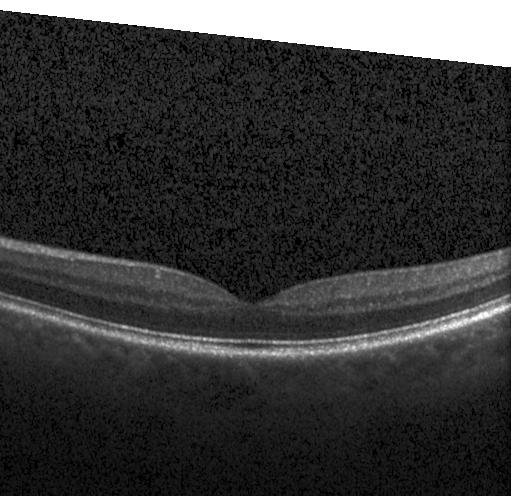
Centered on the fovea, retinal OCT cross-section — Dx: neither choroidal neovascularization, diabetic macular edema, nor drusen.